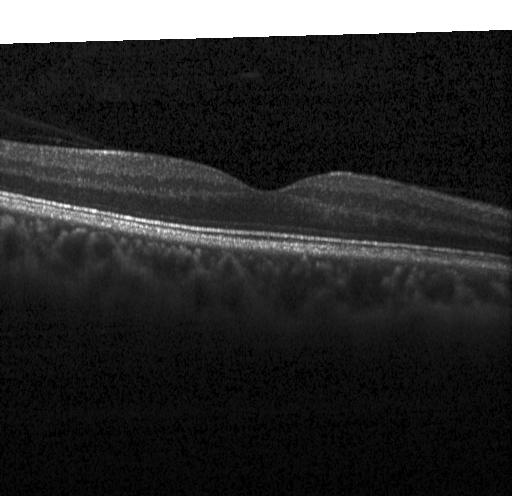
Heidelberg Spectralis; OCT line scan.
This B-scan demonstrates neither choroidal neovascularization, diabetic macular edema, nor drusen.